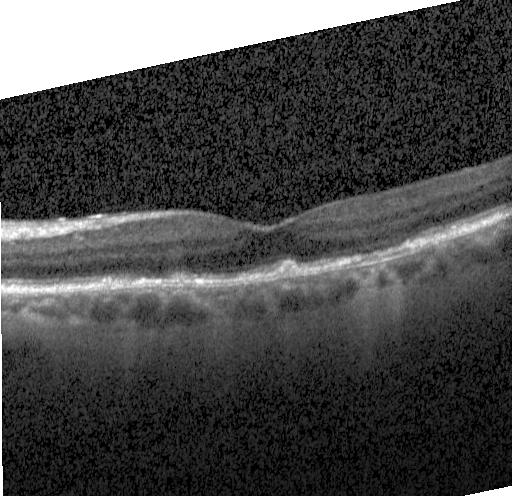
Finding: drusen.